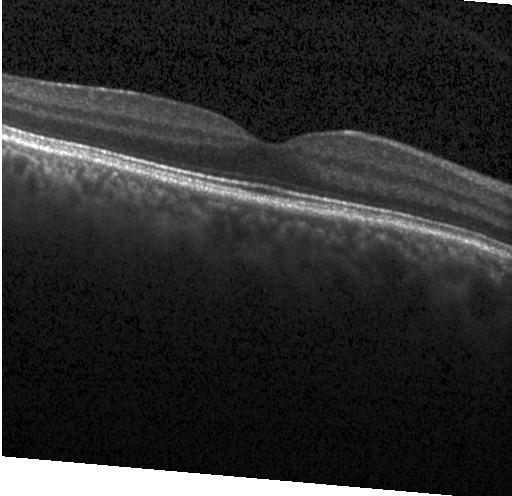

Horizontal scan through the fovea · optical coherence tomography B-scan · spectral-domain OCT
Dx: no evidence of CNV, DME, or drusen.